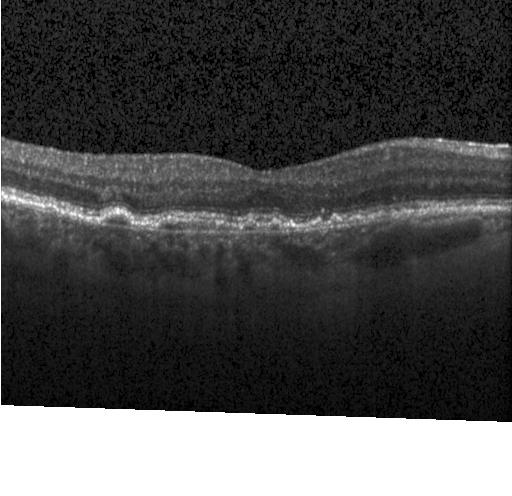
OCT scan showing CNV.